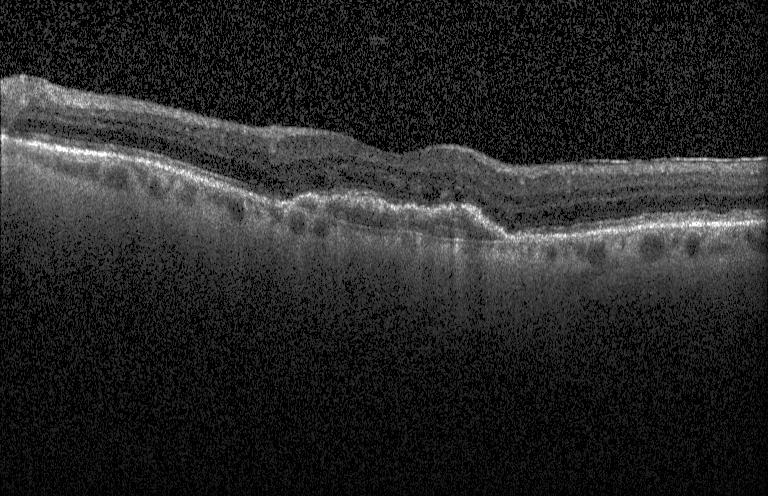 Horizontal scan through the fovea, retinal OCT B-scan, spectral-domain OCT. This B-scan demonstrates a choroidal neovascular membrane.